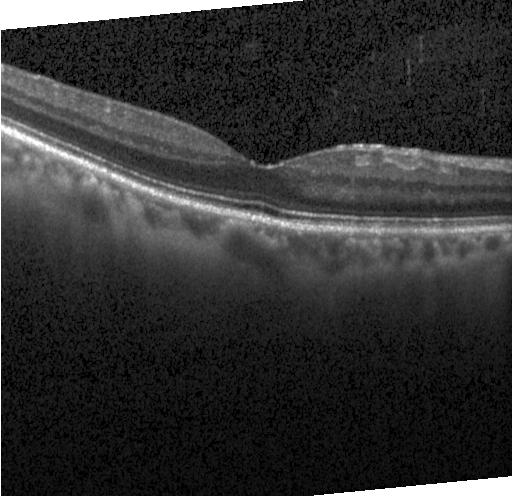

OCT B-scan showing no evidence of choroidal neovascularization, diabetic macular edema, or drusen.